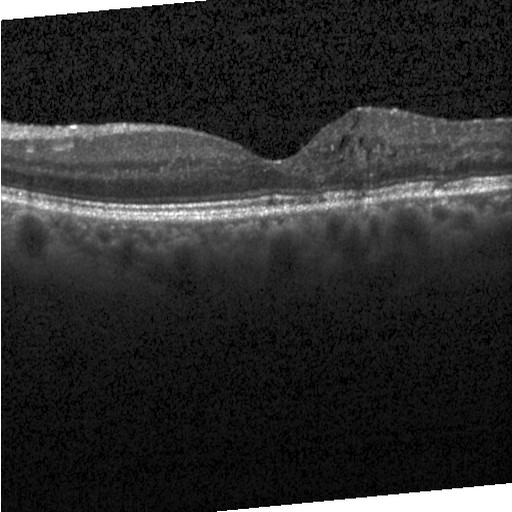 Diabetic macular edema.